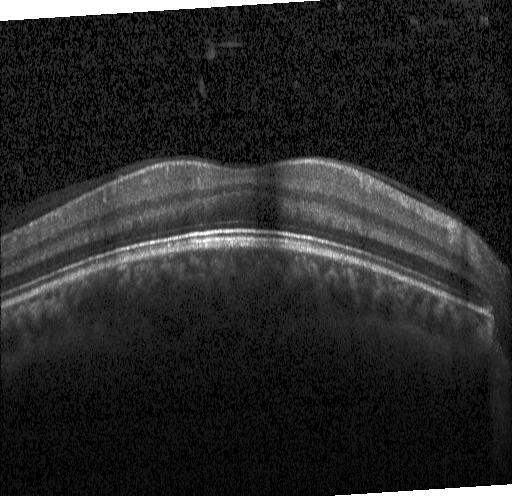

Retinal OCT B-scan — Dx: no CNV, no DME, and no drusen.